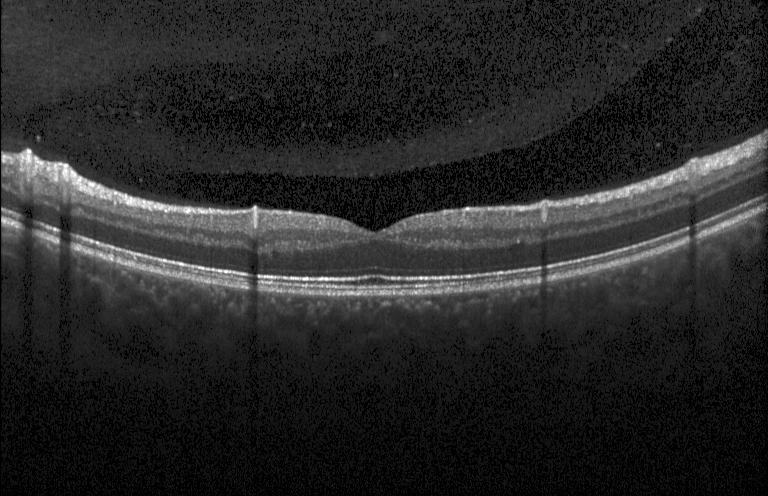
OCT B-scan.
Impression: neither CNV, DME, nor drusen.